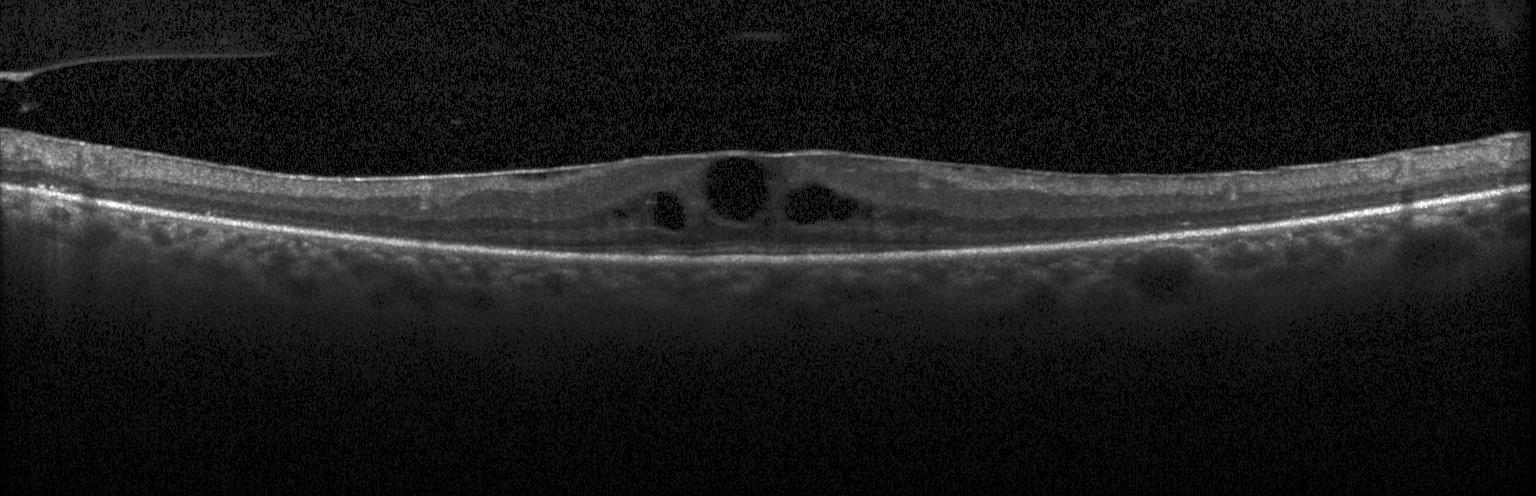
Macular OCT: diabetic macular edema (DME).